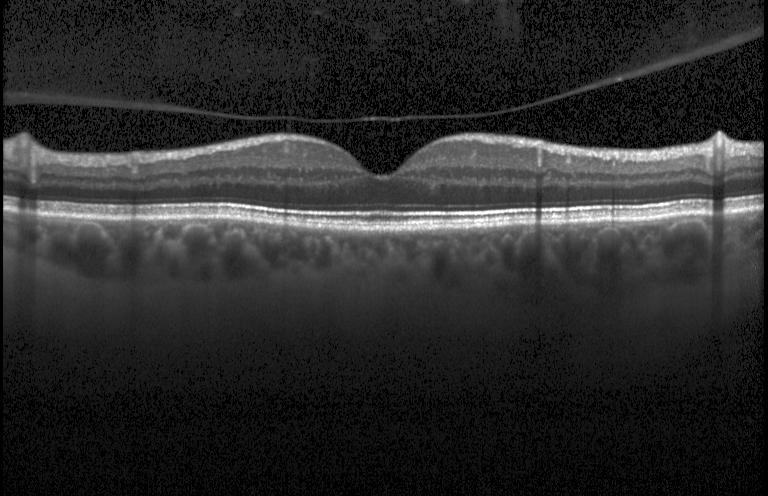
This B-scan demonstrates no CNV, no DME, and no drusen.